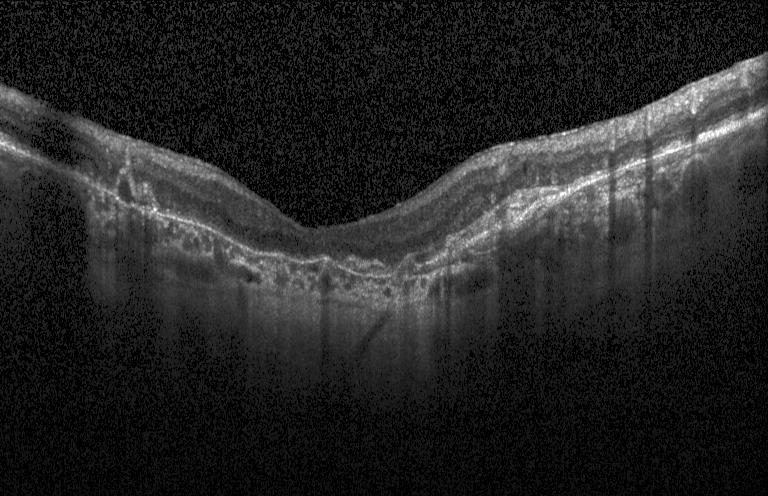
Heidelberg Spectralis OCT system · retinal OCT cross-section · SD-OCT — Assessment: choroidal neovascularization (CNV).